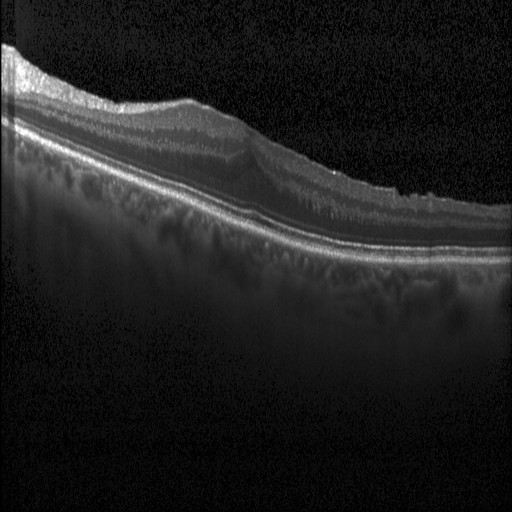
Centered on the fovea, Heidelberg Spectralis OCT system, spectral-domain OCT, OCT B-scan
Impression: diabetic macular edema (DME).